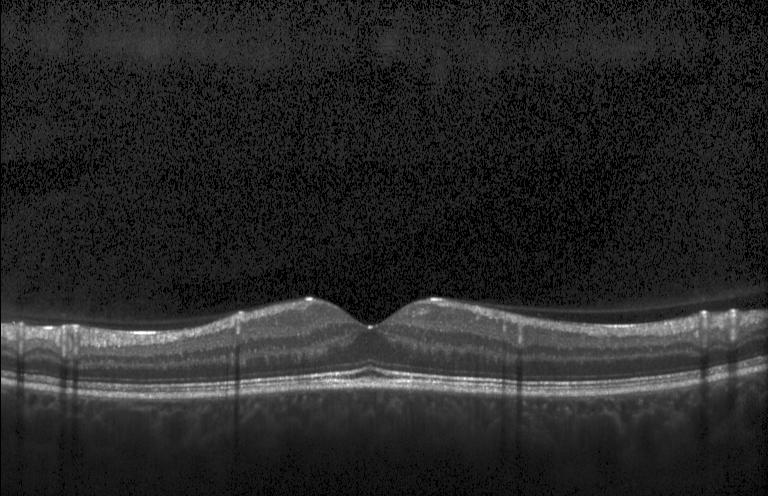
OCT B-scan
Finding: no evidence of choroidal neovascularization, diabetic macular edema, or drusen.